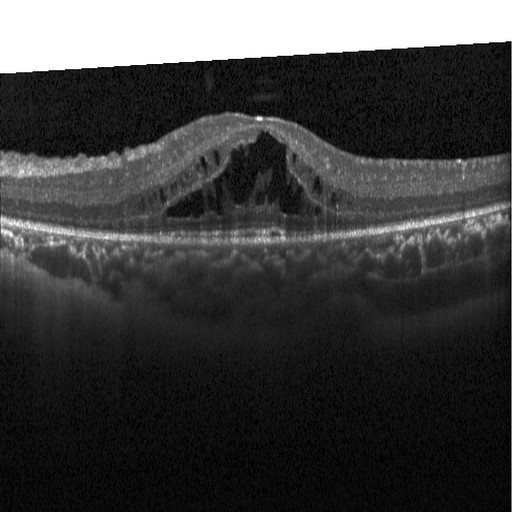

Spectral-domain optical coherence tomography, optical coherence tomography scan, fovea-centered, acquired on a Heidelberg Spectralis
Assessment: diabetic macular edema (DME).